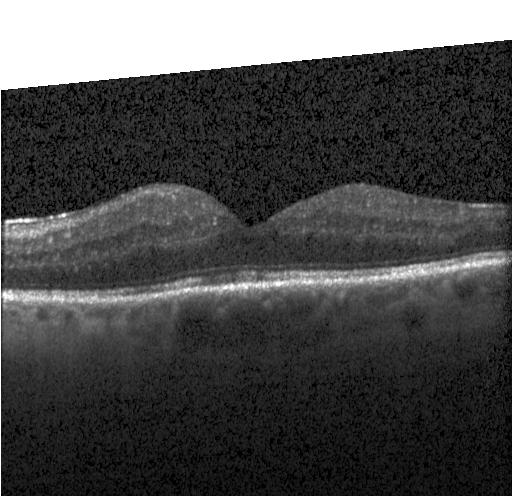

Optical coherence tomography scan.
Impression: no evidence of choroidal neovascularization, diabetic macular edema, or drusen.